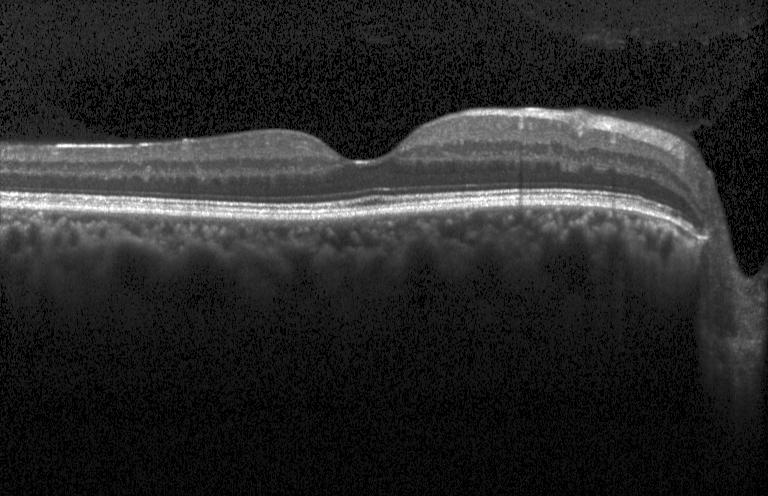
OCT B-scan · acquired on a Heidelberg Spectralis · through the macula.
No choroidal neovascularization, diabetic macular edema, or drusen.